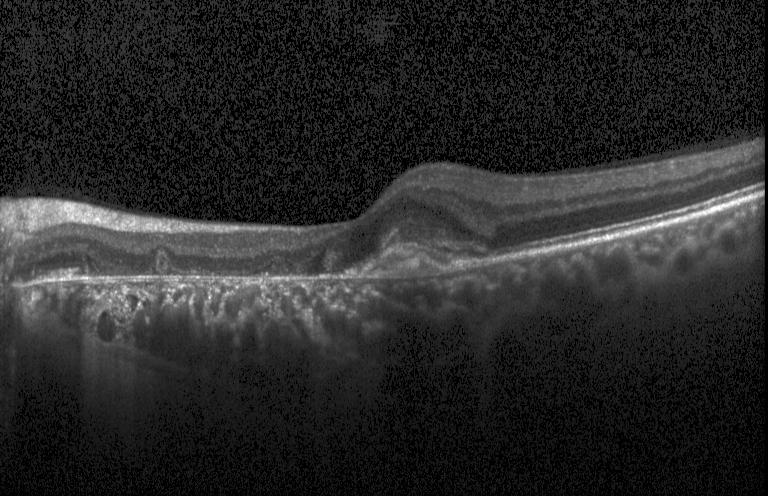
Retinal OCT B-scan · fovea-centered — Dx: CNV.